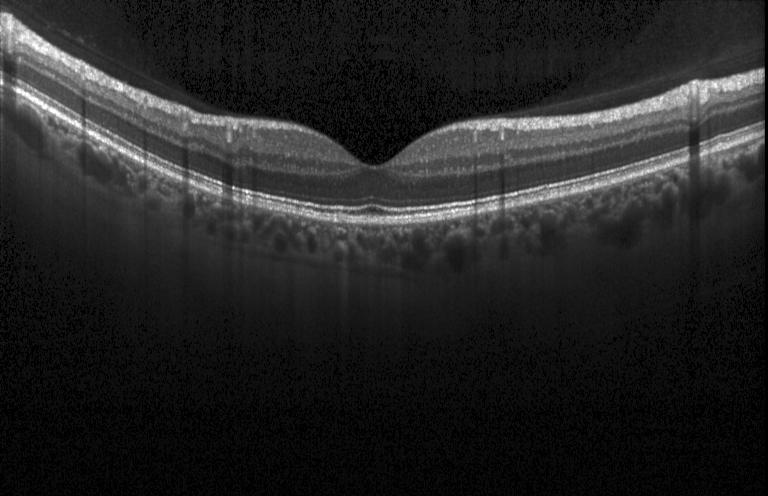 Centered on the fovea · OCT line scan — Diagnosis: no CNV, no DME, and no drusen.